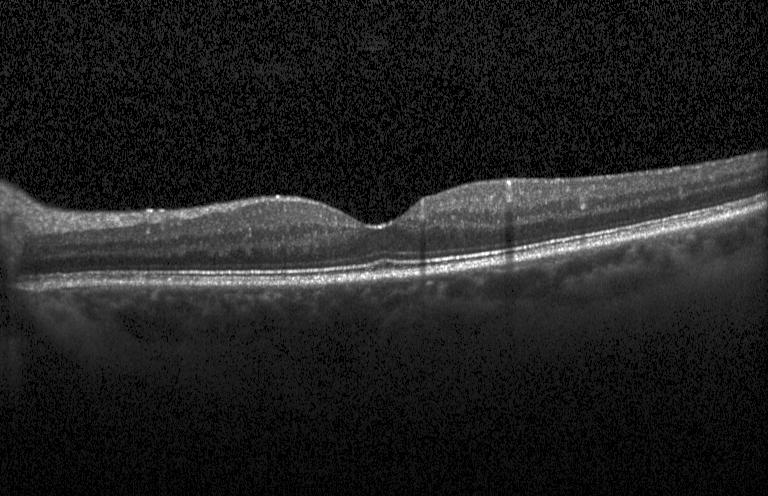
OCT line scan · through the macula.
Diagnosis: neither choroidal neovascularization, diabetic macular edema, nor drusen.